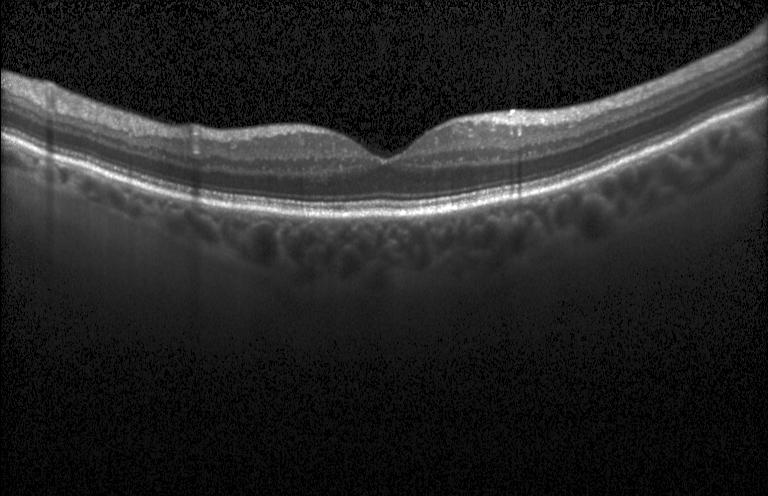

Finding: no choroidal neovascularization, no diabetic macular edema, and no drusen.